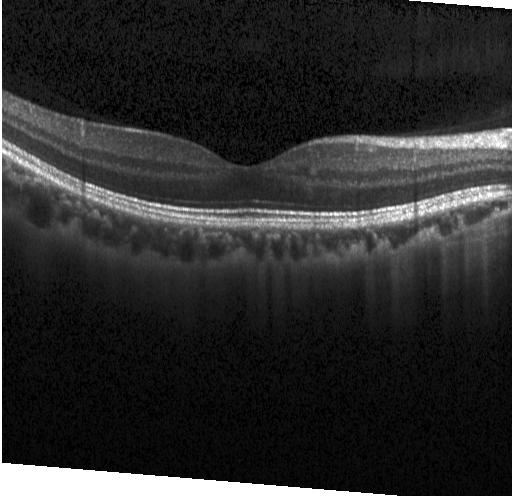
Horizontal scan through the fovea. SD-OCT. Optical coherence tomography scan. This B-scan demonstrates neither choroidal neovascularization, diabetic macular edema, nor drusen.